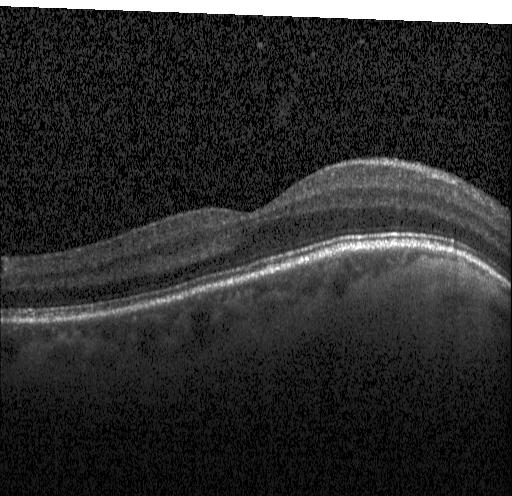
SD-OCT; retinal OCT B-scan.
Assessment: neither choroidal neovascularization, diabetic macular edema, nor drusen.